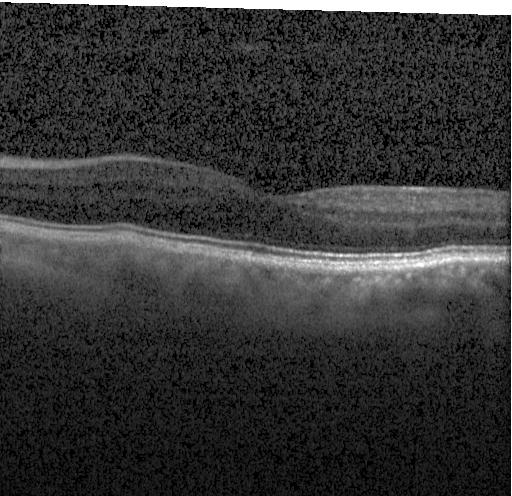
Optical coherence tomography scan — Finding: neither CNV, DME, nor drusen.